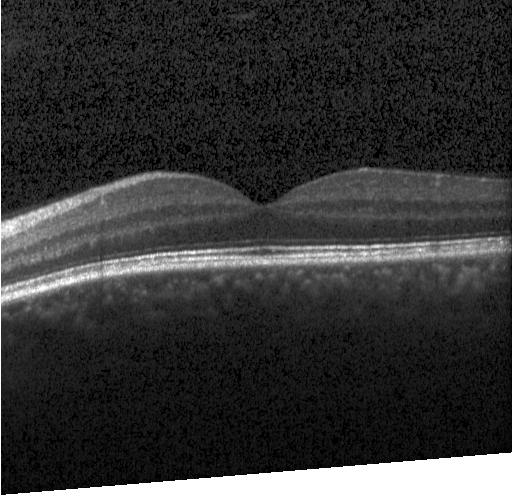
Retinal OCT cross-section.
Diagnosis: no choroidal neovascularization, diabetic macular edema, or drusen.